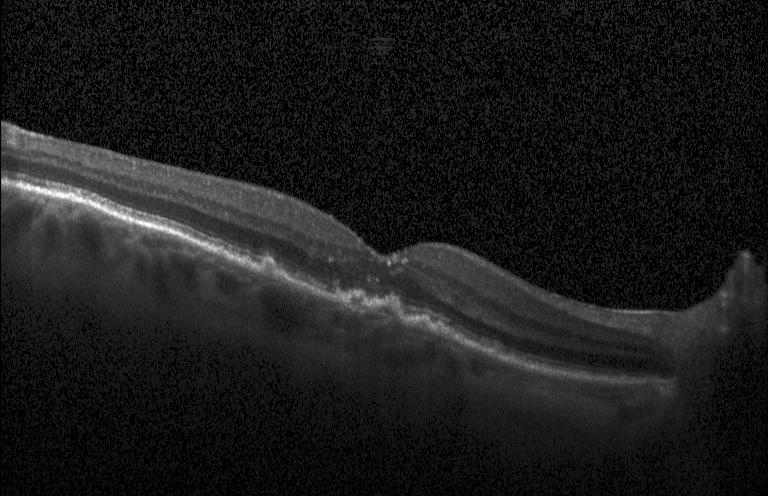
Dx: sub-RPE drusenoid deposits.